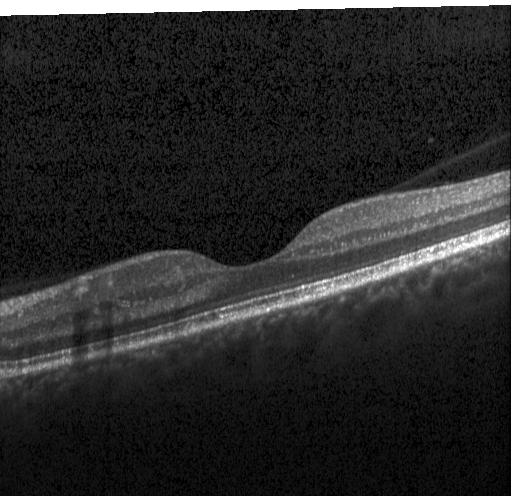 Optical coherence tomography B-scan.
Diagnosis: no evidence of CNV, DME, or drusen.